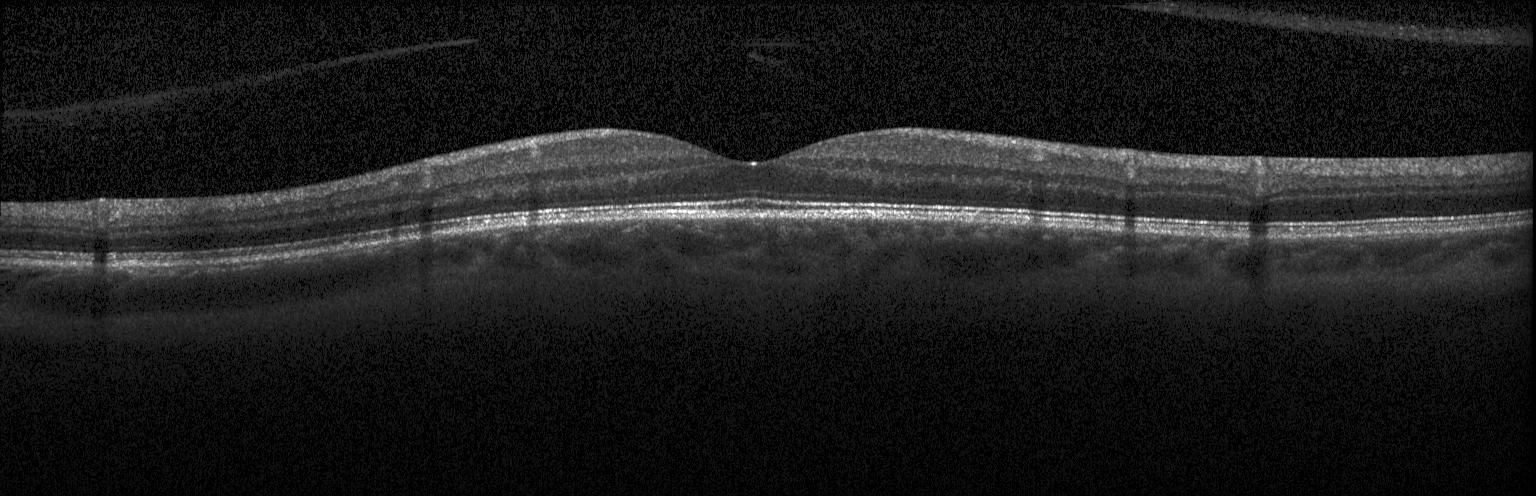 Optical coherence tomography B-scan. Macular OCT: no choroidal neovascularization, no diabetic macular edema, and no drusen.